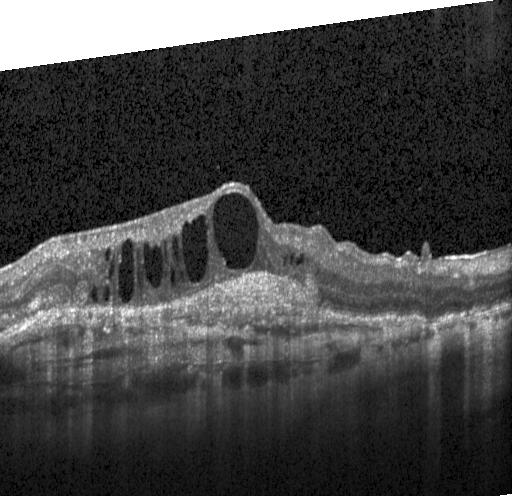

OCT scan showing choroidal neovascularization (CNV).